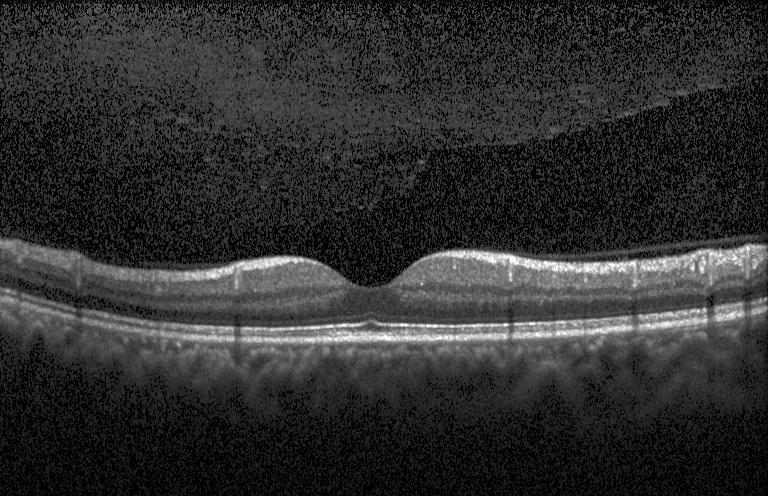 Spectral-domain OCT B-scan: neither CNV, DME, nor drusen.